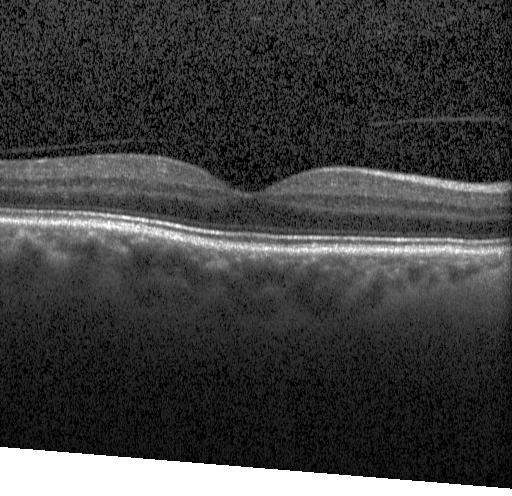
Diagnosis: no CNV, no DME, and no drusen.